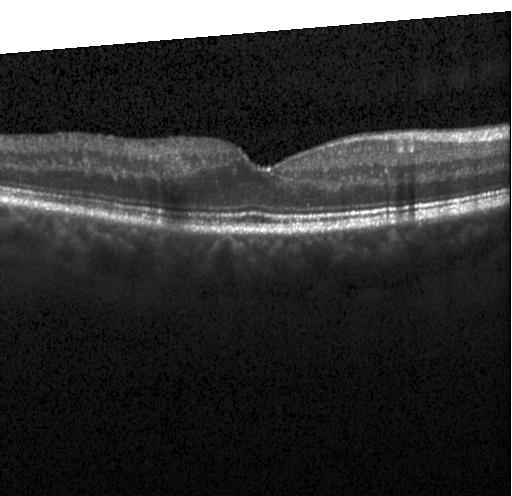 Acquired on a Heidelberg Spectralis. OCT B-scan.
OCT finding: no evidence of choroidal neovascularization, diabetic macular edema, or drusen.